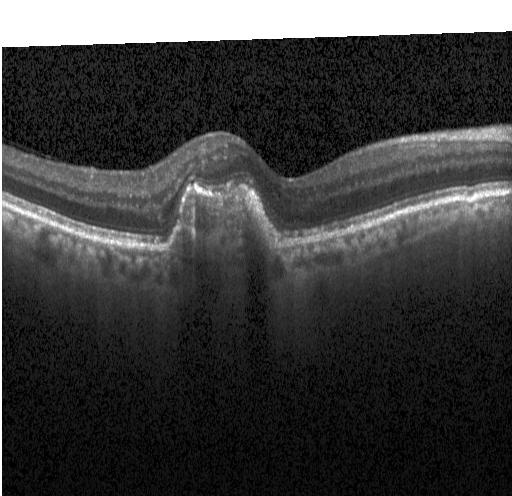 Acquired on a Heidelberg Spectralis, optical coherence tomography B-scan
OCT finding: a choroidal neovascular membrane.